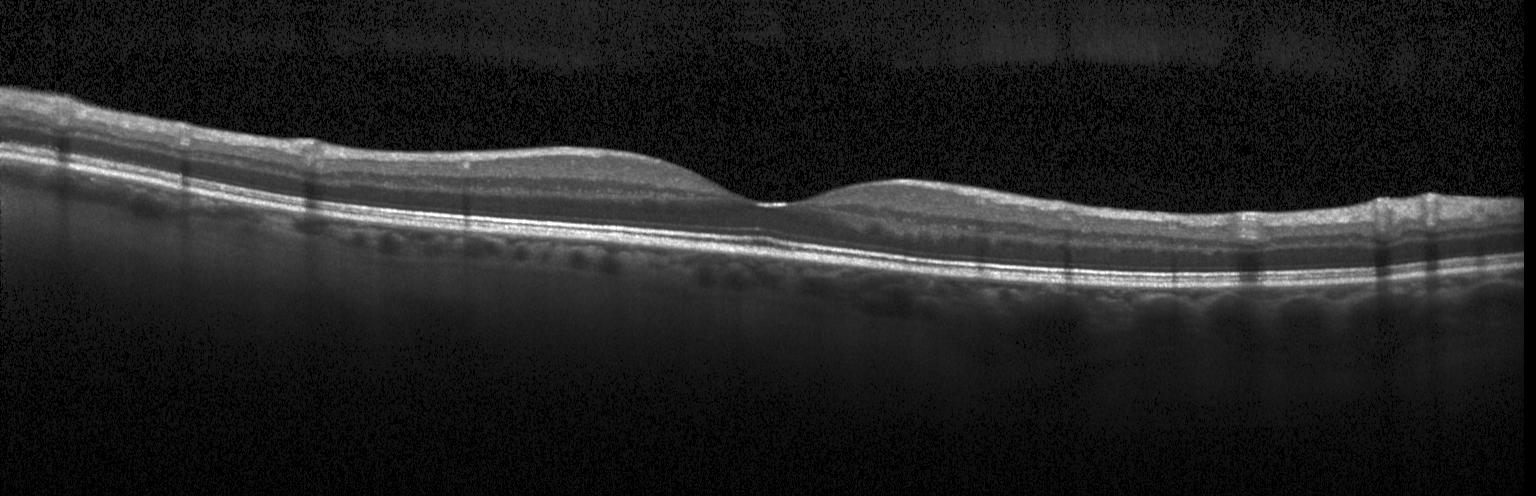

Retinal OCT B-scan.
This B-scan demonstrates neither choroidal neovascularization, diabetic macular edema, nor drusen.